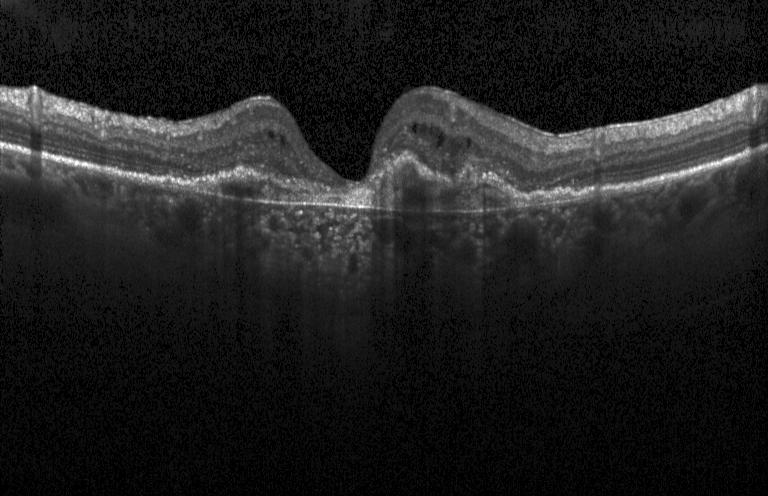 Heidelberg Spectralis. Horizontal scan through the fovea. Retinal OCT cross-section. Spectral-domain OCT. Diagnosis: a choroidal neovascular membrane.